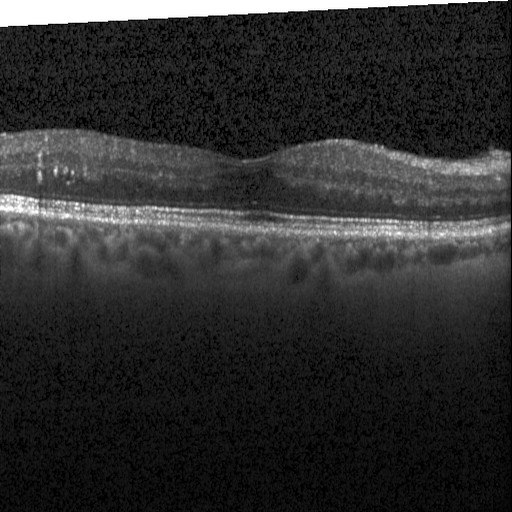

Instrument: Heidelberg Spectralis, retinal OCT B-scan, fovea-centered — Diagnosis: diabetic macular edema (DME).